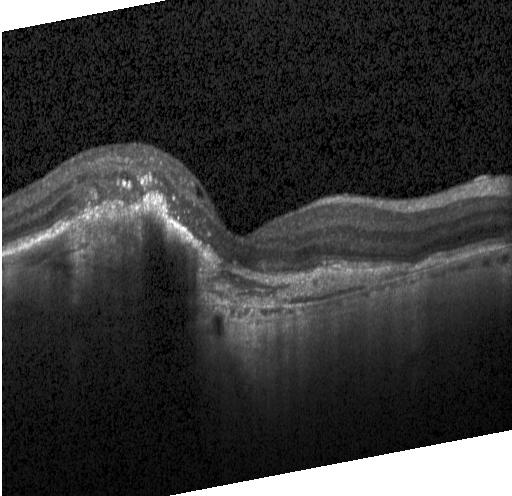 Retinal OCT cross-section · horizontal scan through the fovea · spectral-domain optical coherence tomography · instrument: Heidelberg Spectralis.
Macular OCT: choroidal neovascularization (CNV).